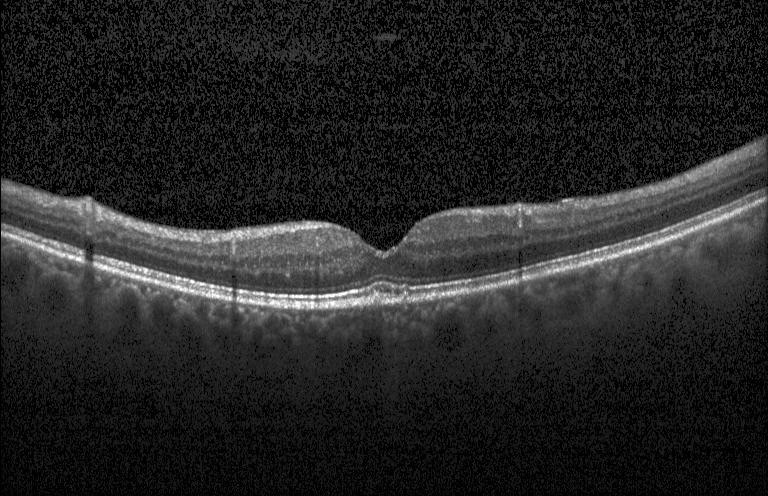 Acquired on a Heidelberg Spectralis; retinal OCT B-scan; spectral-domain OCT; macular scan.
The scan shows no CNV, no DME, and no drusen.